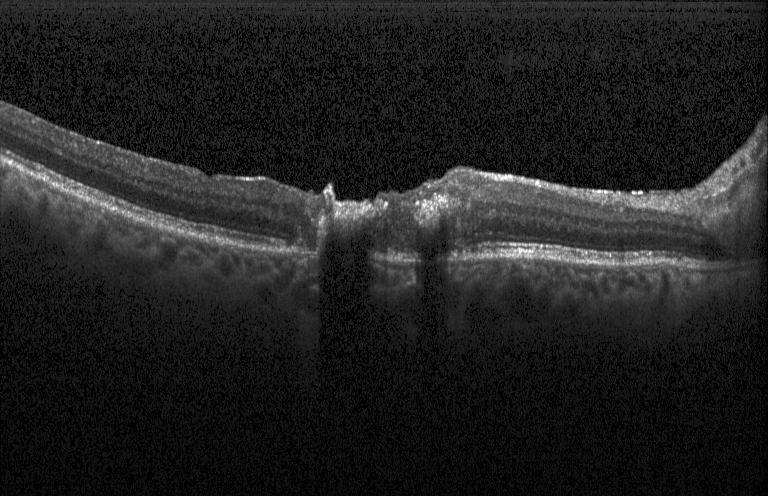
Retinal OCT cross-section. Impression: choroidal neovascularization (CNV).